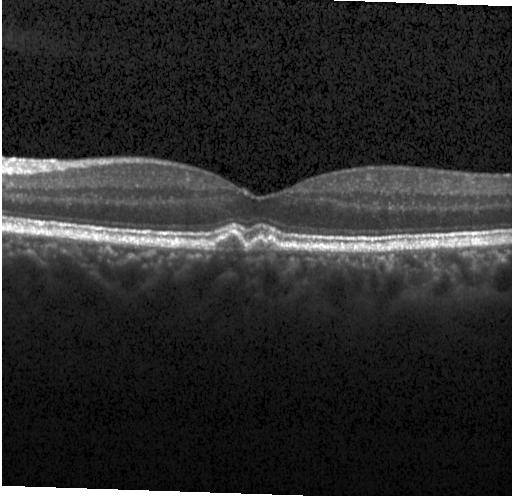
Macular OCT: multiple drusen.